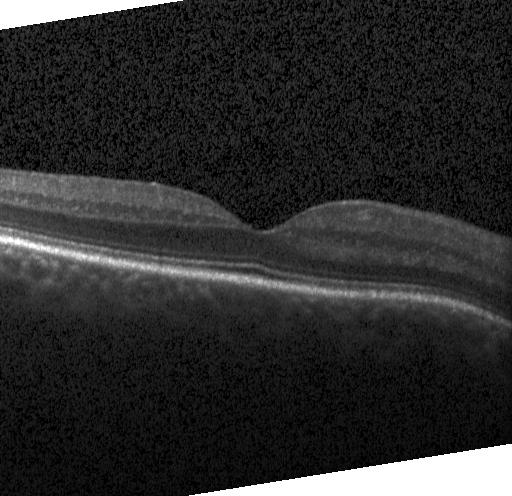
Assessment: no choroidal neovascularization, no diabetic macular edema, and no drusen.